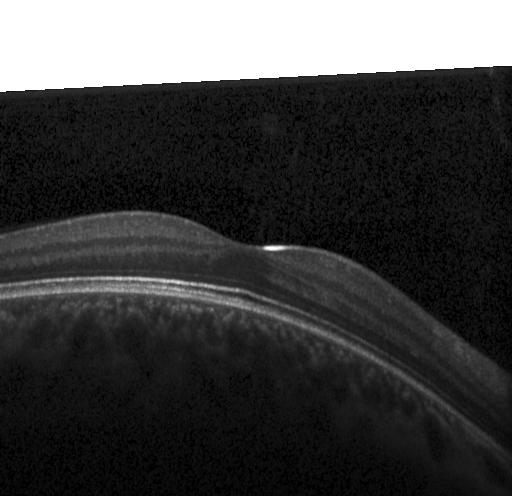
Retinal OCT B-scan, through the macula, spectral-domain OCT, Heidelberg Spectralis OCT system
OCT finding: neither CNV, DME, nor drusen.